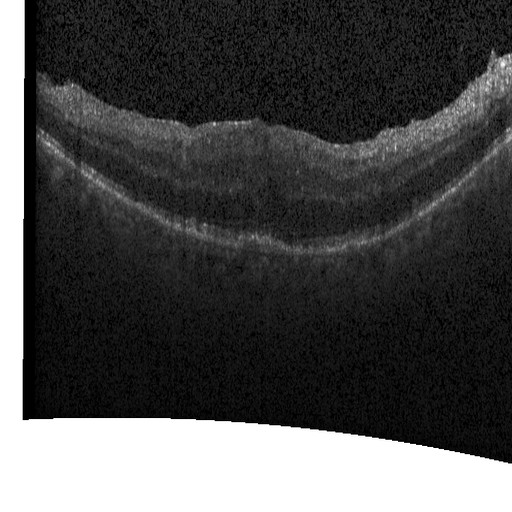
Retinal OCT cross-section.
Diagnosis: diabetic macular edema.